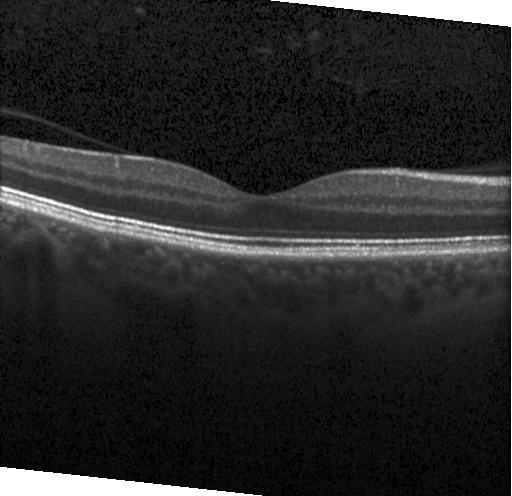
No CNV, DME, or drusen.